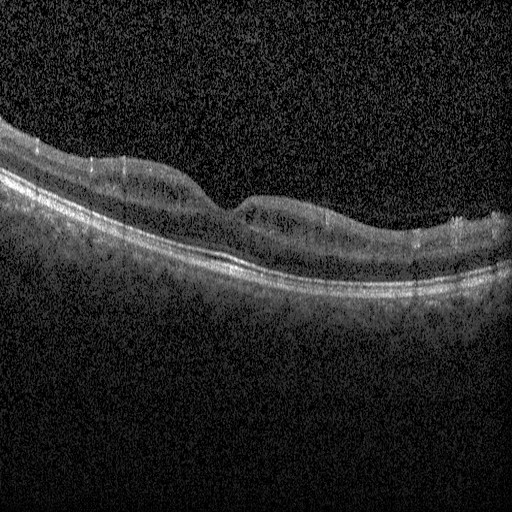

Finding: diabetic macular edema (DME).